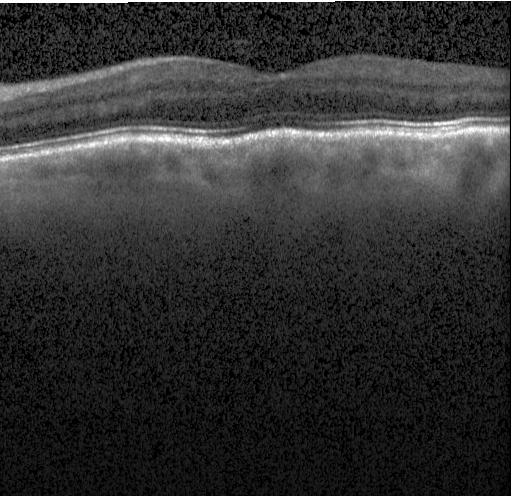
OCT line scan. Assessment: no CNV, DME, or drusen.